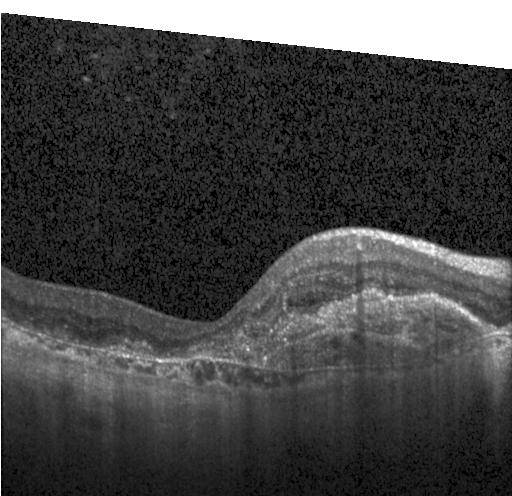

SD-OCT; retinal OCT cross-section; macular scan — This B-scan demonstrates choroidal neovascularization.